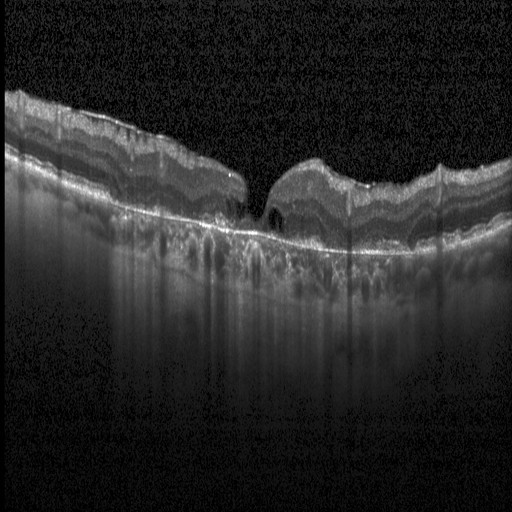 OCT line scan. Spectral-domain optical coherence tomography.
Impression: diabetic macular edema (DME).